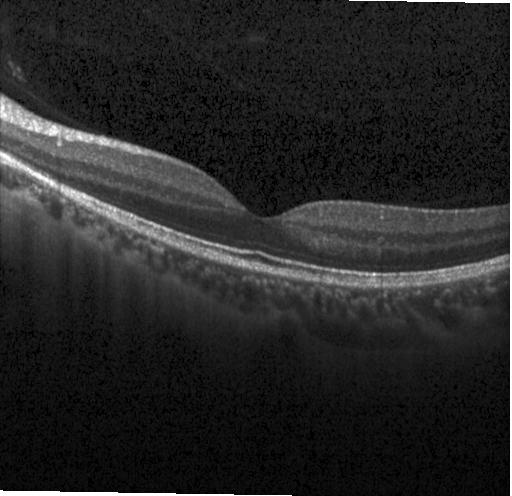

Retinal OCT B-scan · spectral-domain optical coherence tomography · through the macula · Heidelberg Spectralis OCT system. Finding: neither choroidal neovascularization, diabetic macular edema, nor drusen.